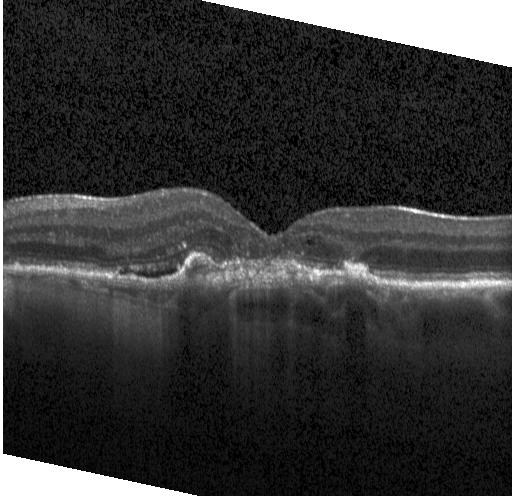

Macular OCT: a choroidal neovascular membrane.